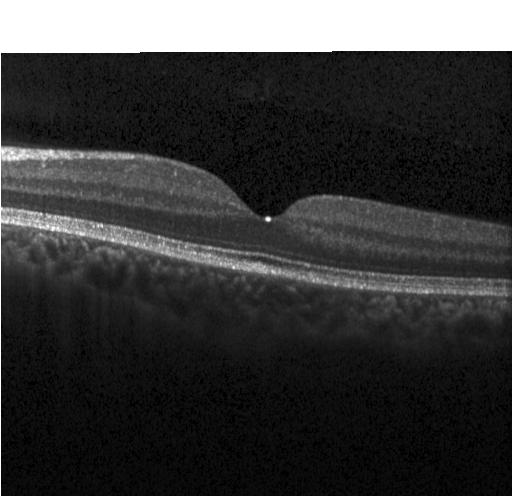 The scan shows neither CNV, DME, nor drusen.